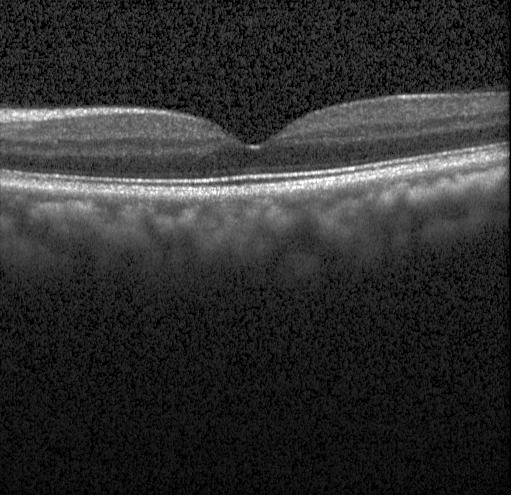 OCT line scan.
Macular OCT: no evidence of choroidal neovascularization, diabetic macular edema, or drusen.